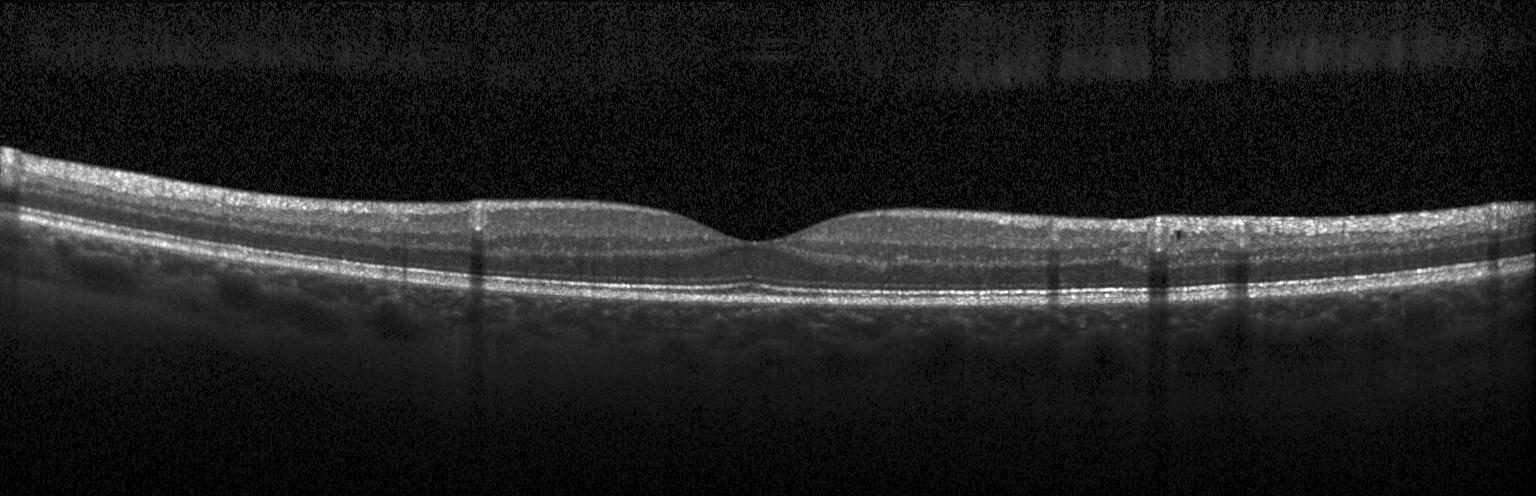
OCT line scan. Diagnosis: neither choroidal neovascularization, diabetic macular edema, nor drusen.